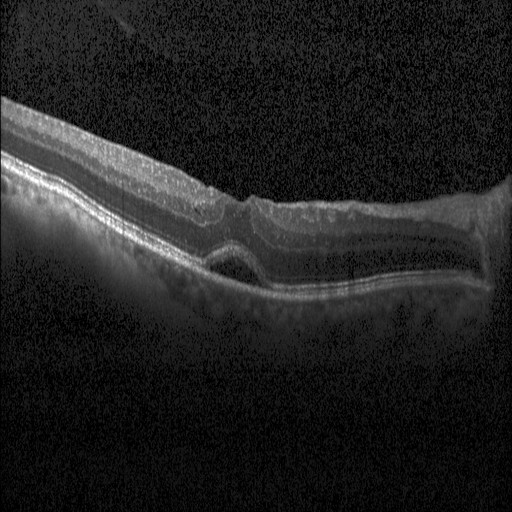
Centered on the fovea, instrument: Heidelberg Spectralis, spectral-domain OCT, optical coherence tomography B-scan — This B-scan demonstrates DME.